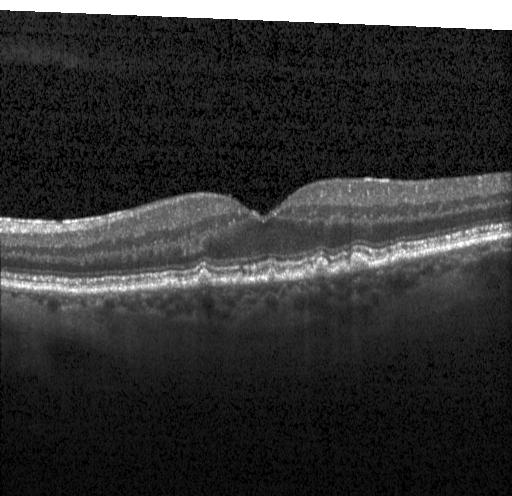

OCT B-scan. Centered on the fovea. Heidelberg Spectralis.
Diagnosis: sub-RPE drusenoid deposits.